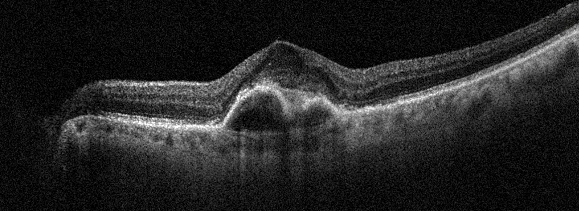
Optical coherence tomography scan, oculus sinister
OCT finding: AMD.